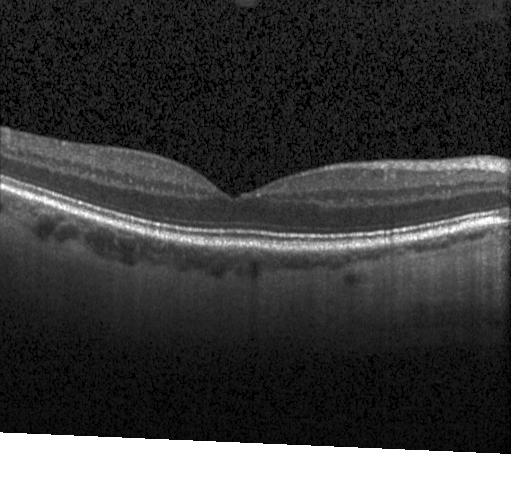

Impression: no evidence of CNV, DME, or drusen.